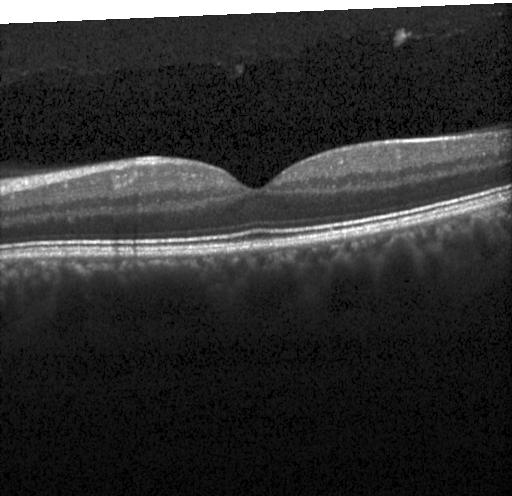

OCT B-scan · through the macula · spectral-domain OCT · instrument: Heidelberg Spectralis. Diagnosis: no choroidal neovascularization, diabetic macular edema, or drusen.